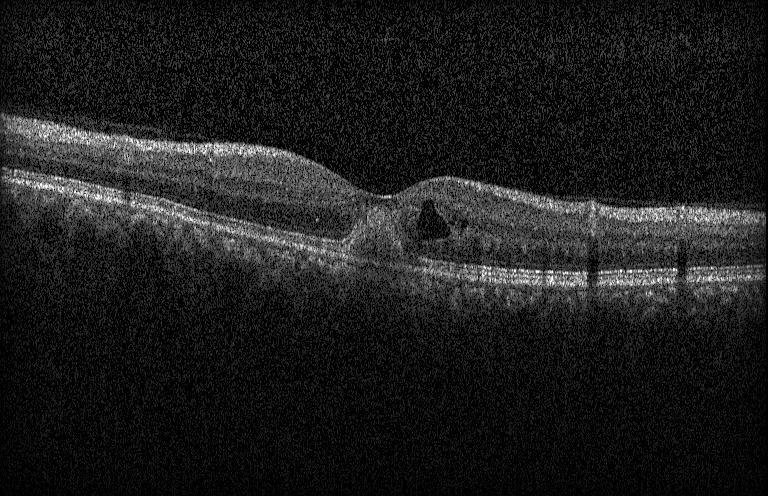 OCT finding: a choroidal neovascular membrane.